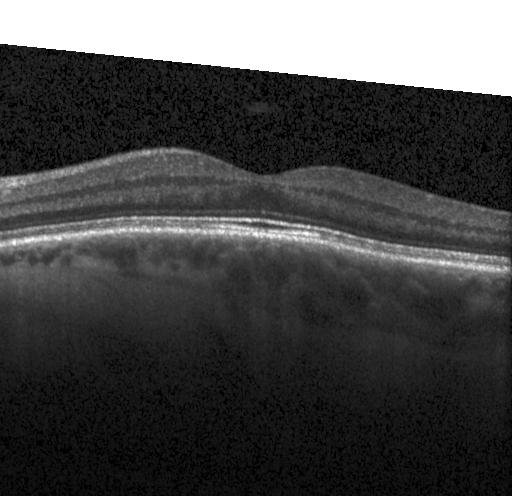 Heidelberg Spectralis OCT system · OCT line scan · SD-OCT.
This B-scan demonstrates no choroidal neovascularization, no diabetic macular edema, and no drusen.